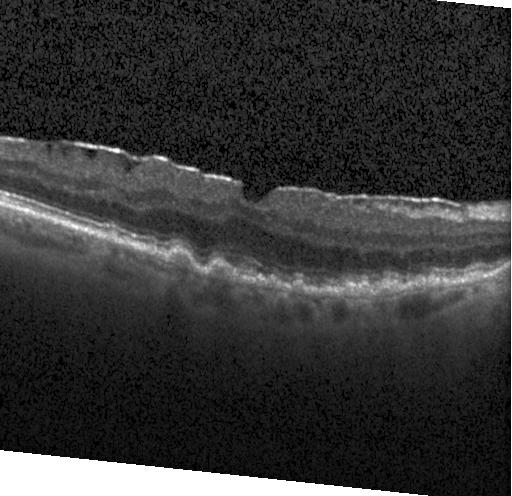

Diagnosis: drusen.